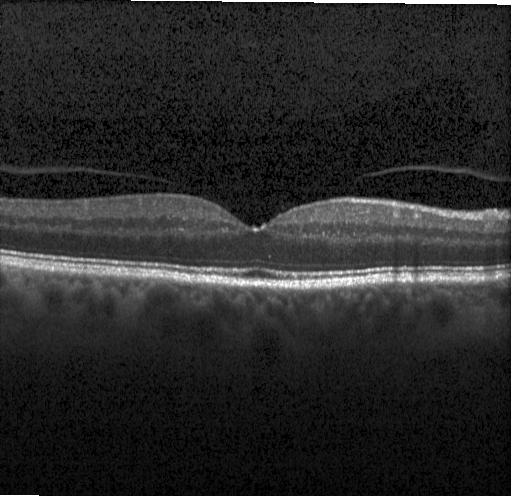

Retinal OCT cross-section.
No choroidal neovascularization, no diabetic macular edema, and no drusen.